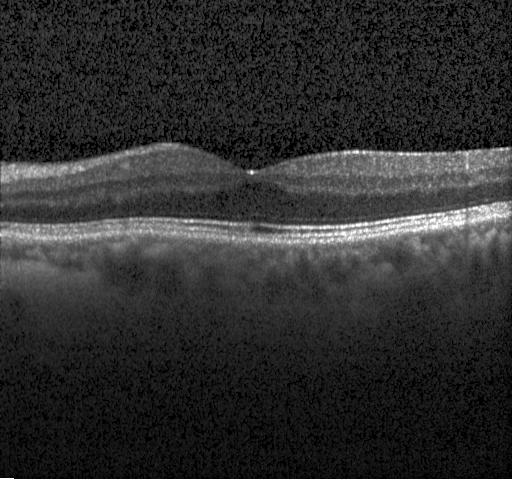 Centered on the fovea; instrument: Heidelberg Spectralis; retinal OCT cross-section
OCT finding: neither choroidal neovascularization, diabetic macular edema, nor drusen.